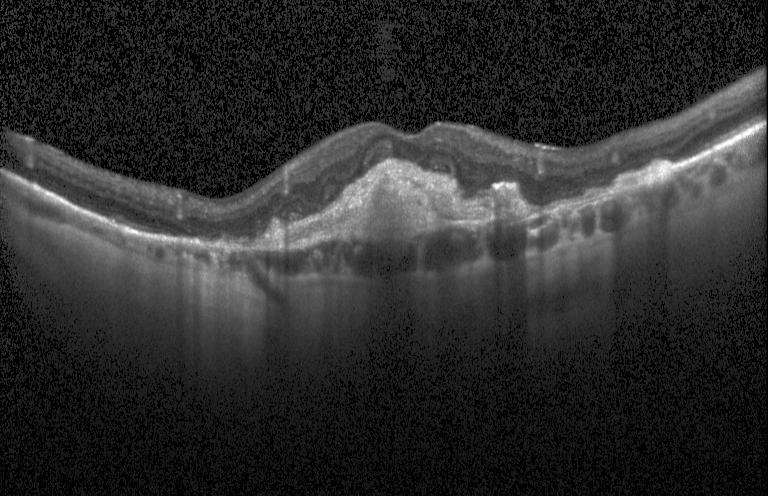

Spectral-domain OCT · optical coherence tomography B-scan · instrument: Heidelberg Spectralis · through the macula
Impression: a choroidal neovascular membrane.